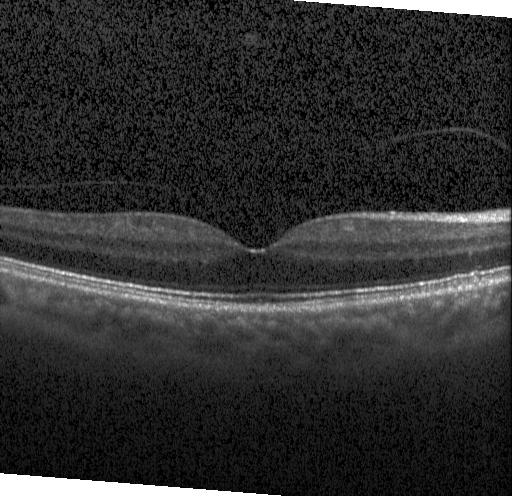 Retinal OCT cross-section · fovea-centered · spectral-domain optical coherence tomography · instrument: Heidelberg Spectralis. Finding: no choroidal neovascularization, diabetic macular edema, or drusen.